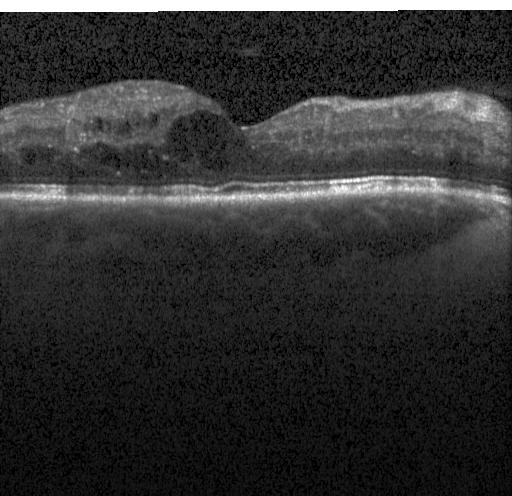
Diagnosis: diabetic macular edema (DME).